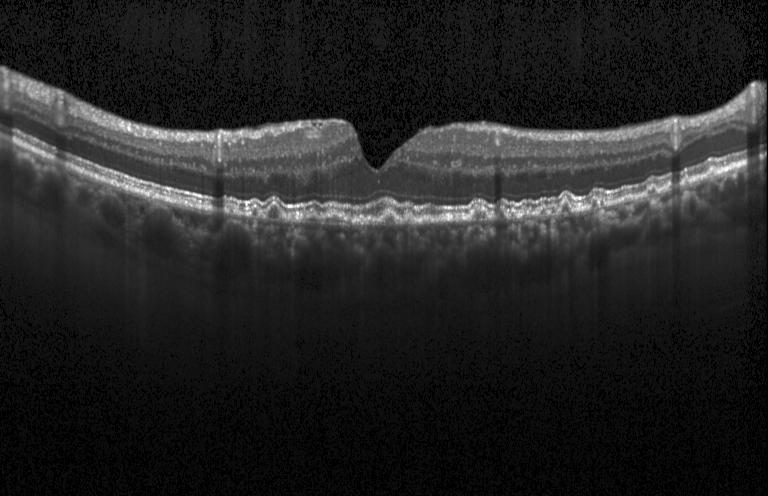

Instrument: Heidelberg Spectralis. OCT line scan. Horizontal scan through the fovea.
Diagnosis: multiple drusen.